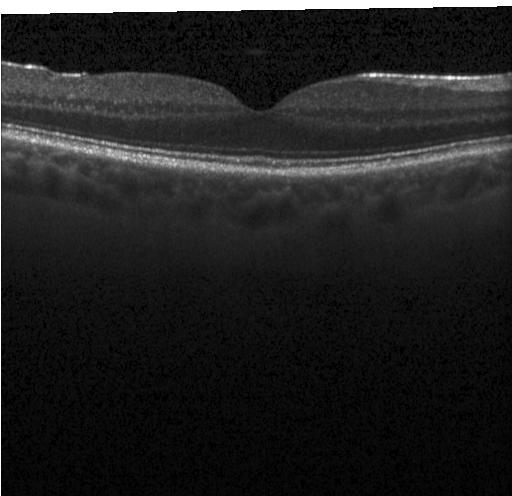

Optical coherence tomography B-scan. The scan shows no choroidal neovascularization, diabetic macular edema, or drusen.